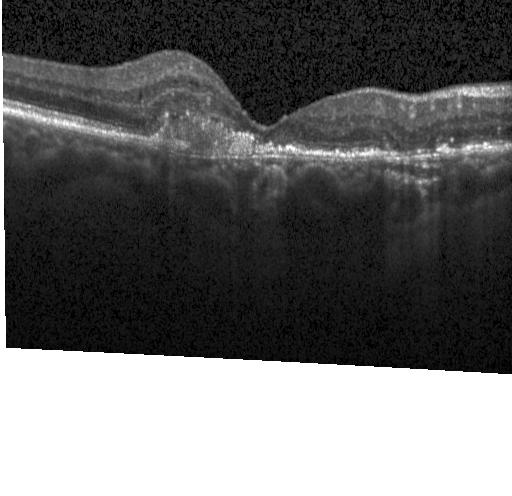

Spectral-domain OCT B-scan: CNV.